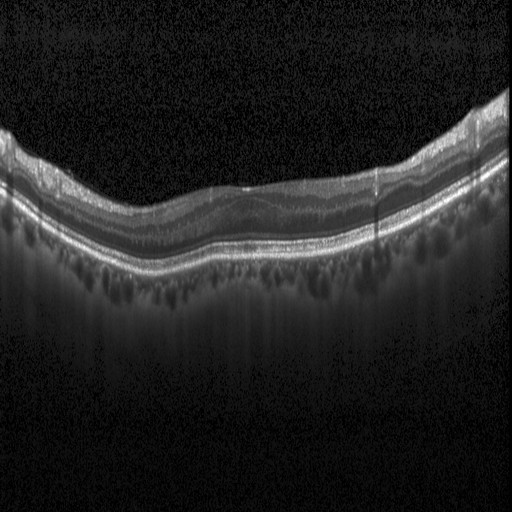 Macular scan · retinal OCT cross-section · spectral-domain optical coherence tomography — The scan shows diabetic macular edema (DME).